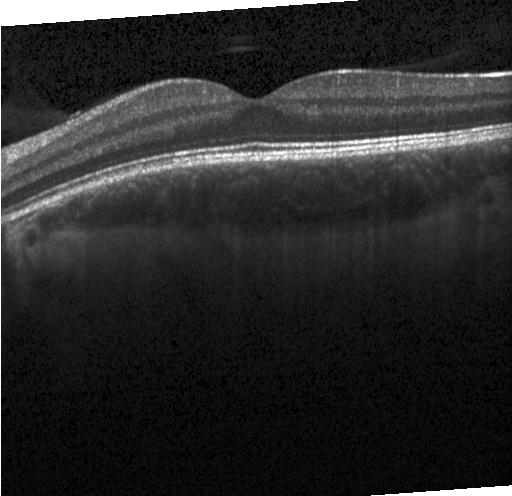

Horizontal scan through the fovea · optical coherence tomography B-scan · spectral-domain OCT.
Dx: no choroidal neovascularization, no diabetic macular edema, and no drusen.